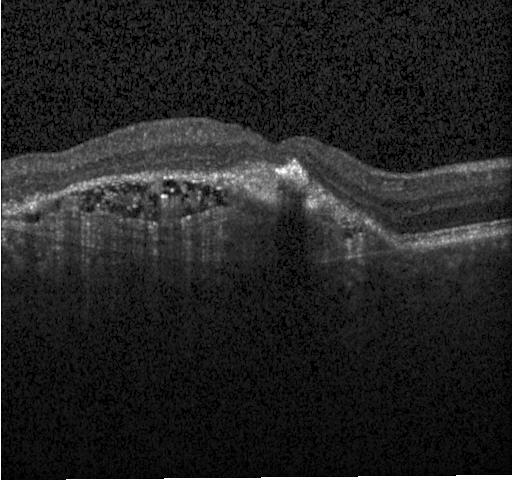
SD-OCT. Retinal OCT B-scan. Heidelberg Spectralis. Through the macula. Choroidal neovascularization (CNV).